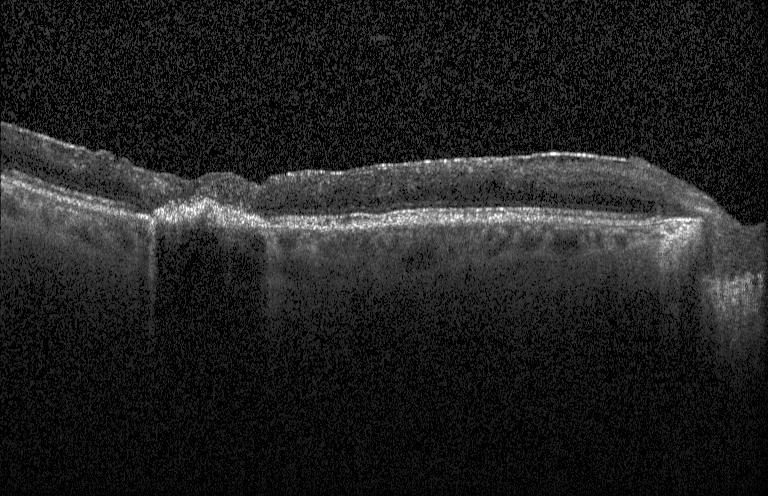 Diagnosis: a choroidal neovascular membrane.